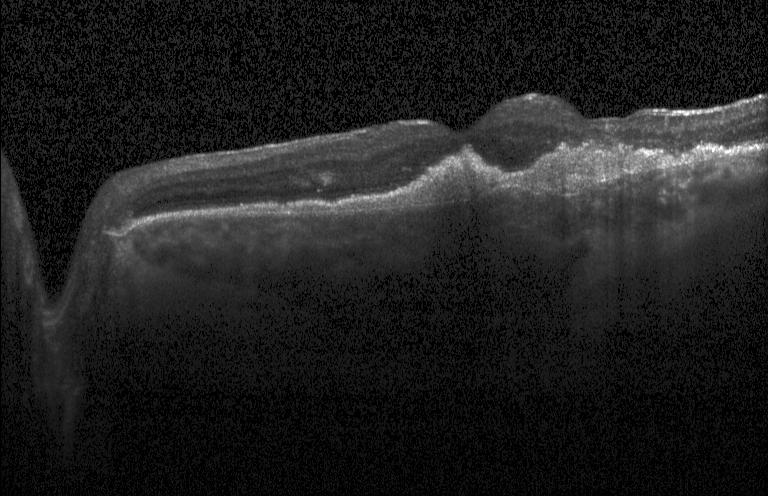
SD-OCT, horizontal scan through the fovea, retinal OCT B-scan — Dx: a choroidal neovascular membrane.